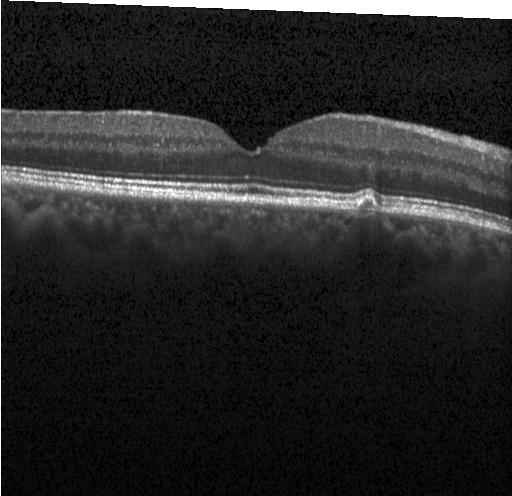
Spectral-domain OCT; optical coherence tomography scan; Heidelberg Spectralis OCT system; horizontal scan through the fovea — This B-scan demonstrates drusen.